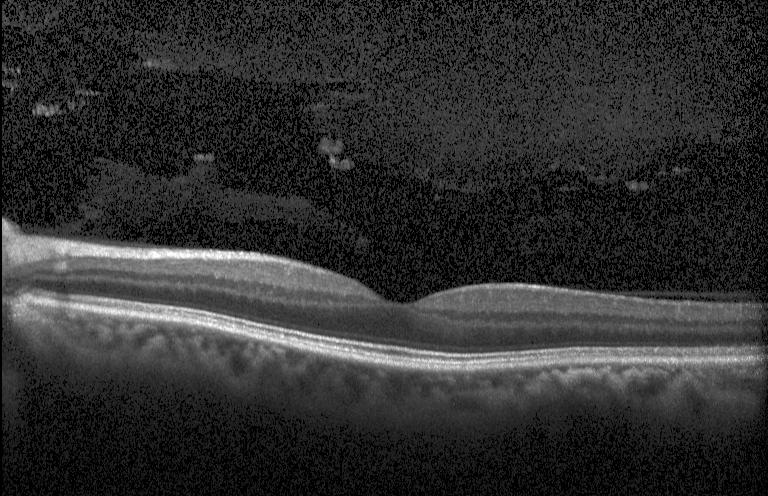
Through the macula. Optical coherence tomography scan. Finding: no evidence of CNV, DME, or drusen.